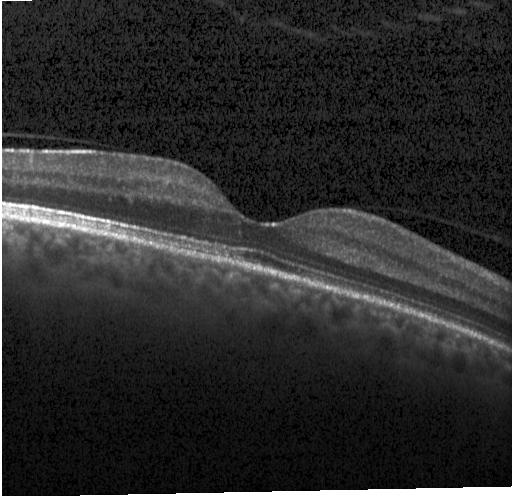
Optical coherence tomography scan, acquired on a Heidelberg Spectralis. Macular OCT: no evidence of CNV, DME, or drusen.